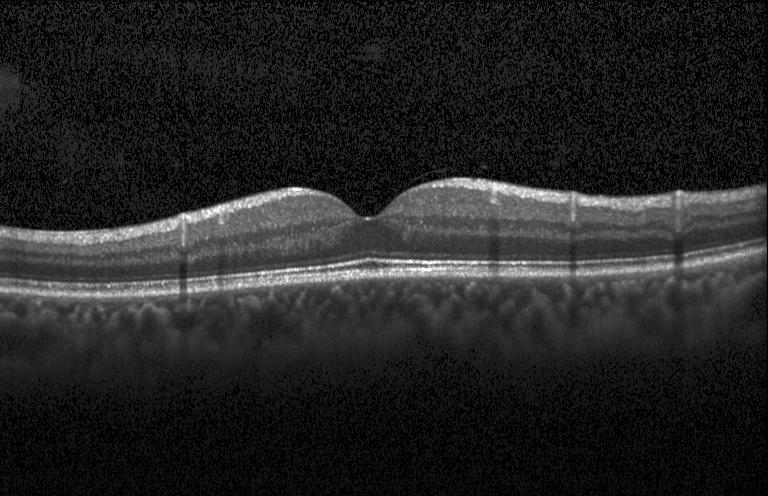 Optical coherence tomography scan
The scan shows neither choroidal neovascularization, diabetic macular edema, nor drusen.